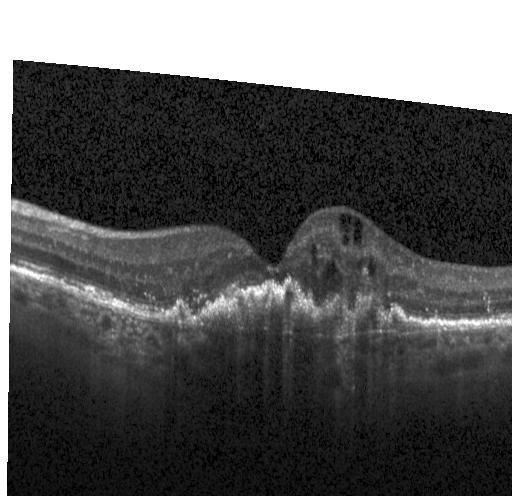 Optical coherence tomography B-scan, Heidelberg Spectralis OCT system, macular scan, spectral-domain optical coherence tomography — A choroidal neovascular membrane.